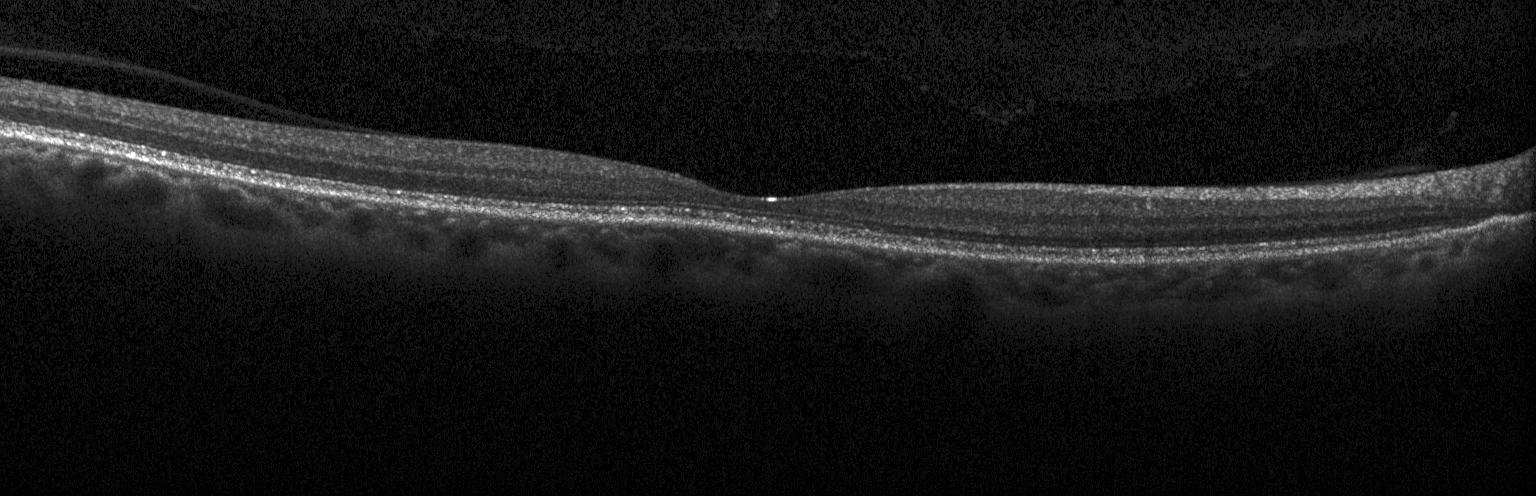
OCT line scan, centered on the fovea. Diagnosis: neither choroidal neovascularization, diabetic macular edema, nor drusen.